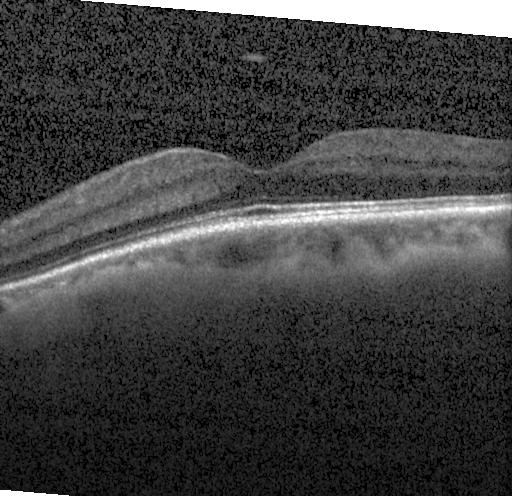

OCT line scan · spectral-domain OCT.
This B-scan demonstrates no evidence of choroidal neovascularization, diabetic macular edema, or drusen.